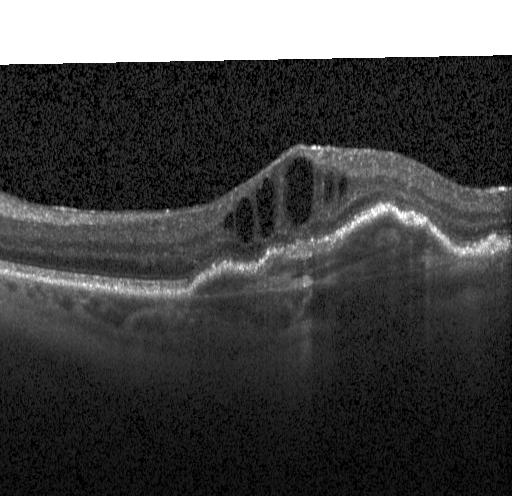

Instrument: Heidelberg Spectralis, SD-OCT, fovea-centered, optical coherence tomography scan.
Diagnosis: a choroidal neovascular membrane.